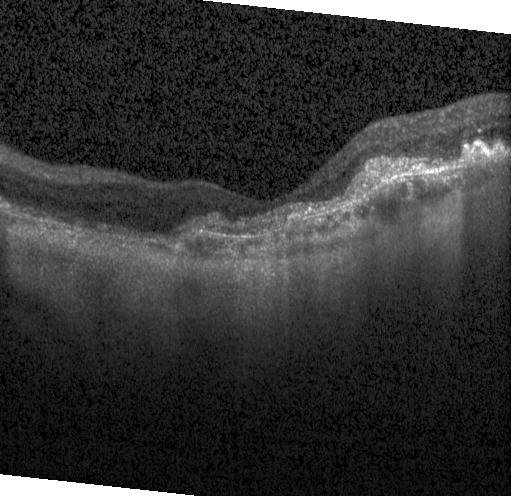 Instrument: Heidelberg Spectralis. Through the macula. SD-OCT. Optical coherence tomography scan. Dx: a choroidal neovascular membrane.